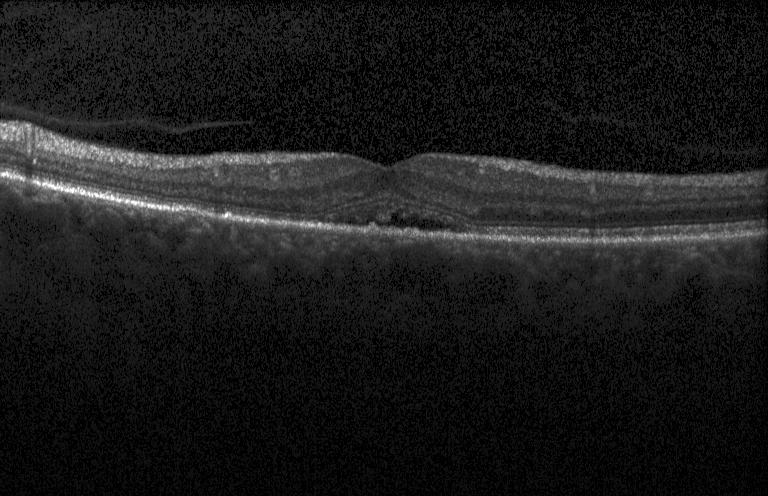

Spectral-domain OCT B-scan: CNV.